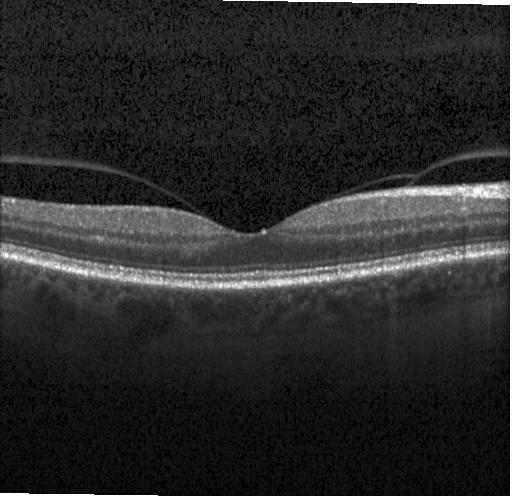

Optical coherence tomography B-scan
Macular OCT: no evidence of choroidal neovascularization, diabetic macular edema, or drusen.